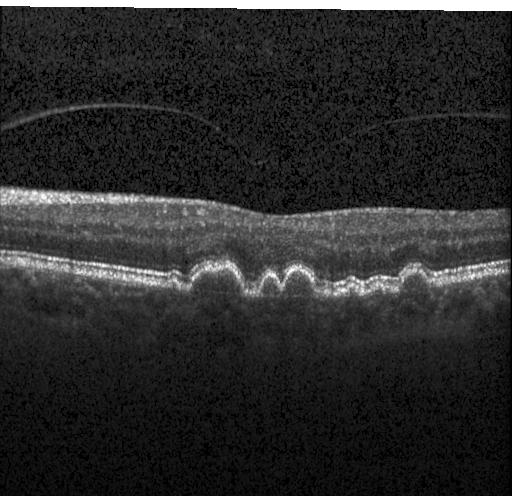 Optical coherence tomography B-scan. Spectral-domain optical coherence tomography.
Impression: drusen.